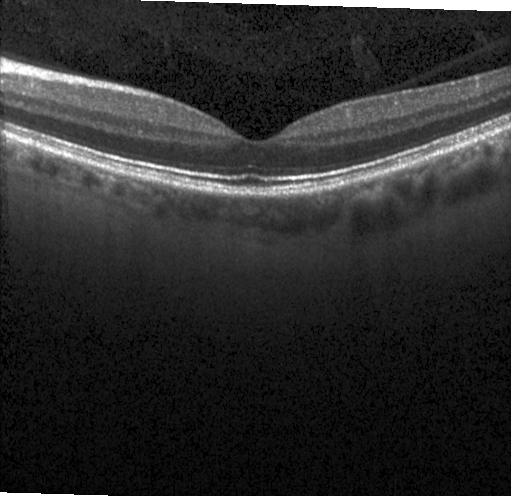

Diagnosis: no choroidal neovascularization, no diabetic macular edema, and no drusen.